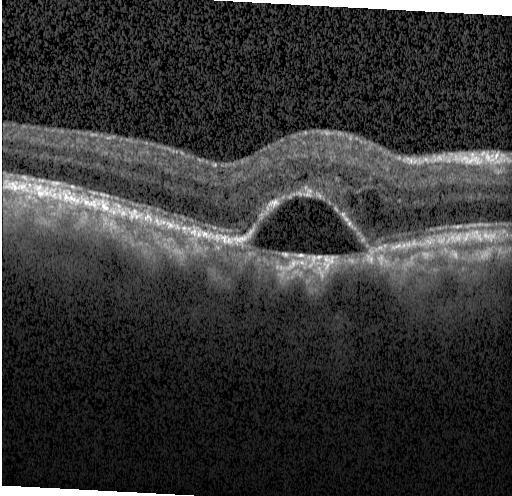 Finding: choroidal neovascularization.